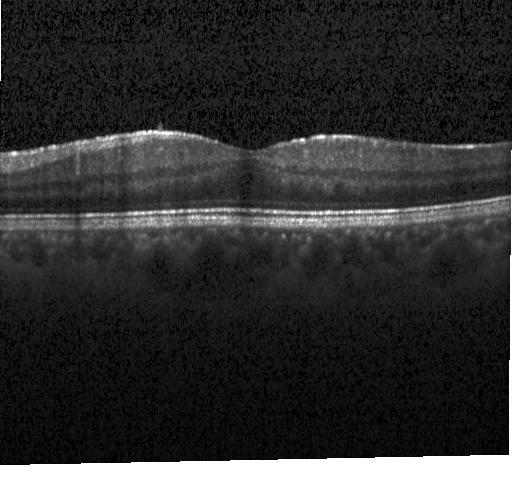 Heidelberg Spectralis. Spectral-domain OCT. OCT B-scan. Through the macula.
This B-scan demonstrates no evidence of choroidal neovascularization, diabetic macular edema, or drusen.